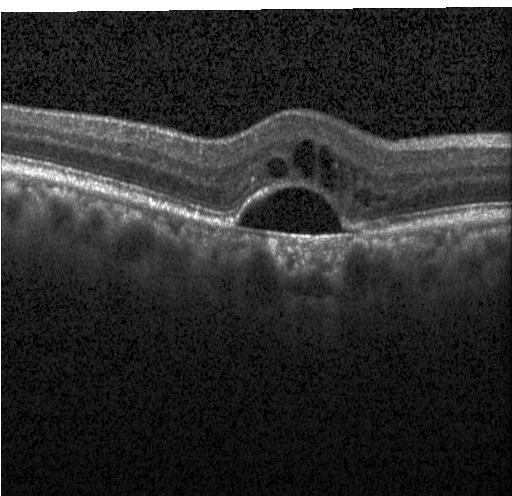

OCT finding: a choroidal neovascular membrane.